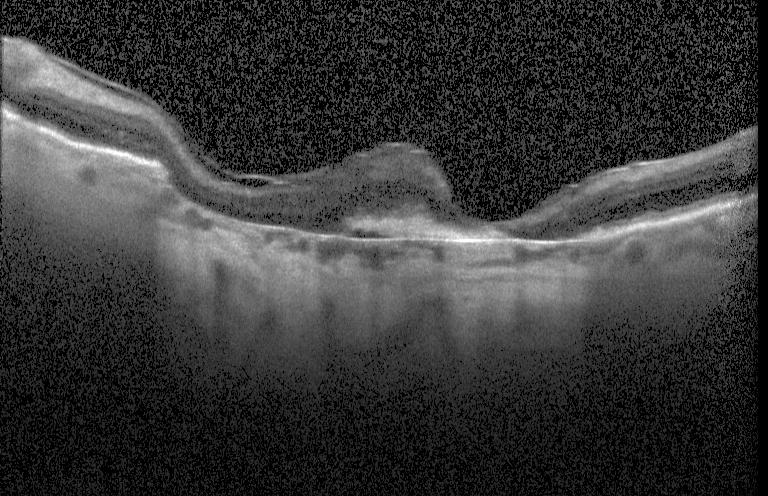
OCT B-scan, acquired on a Heidelberg Spectralis, SD-OCT, horizontal scan through the fovea — The scan shows a choroidal neovascular membrane.